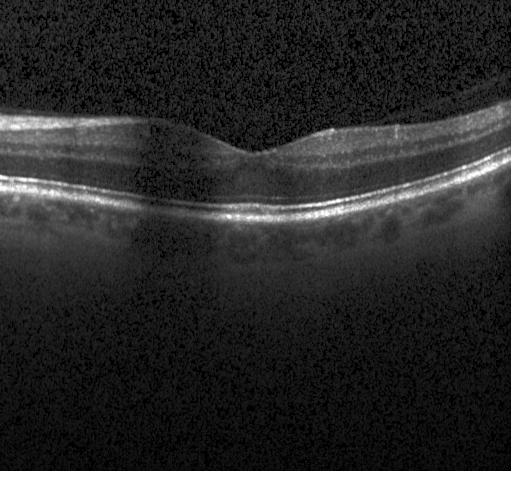

OCT B-scan. Heidelberg Spectralis — Finding: no choroidal neovascularization, diabetic macular edema, or drusen.